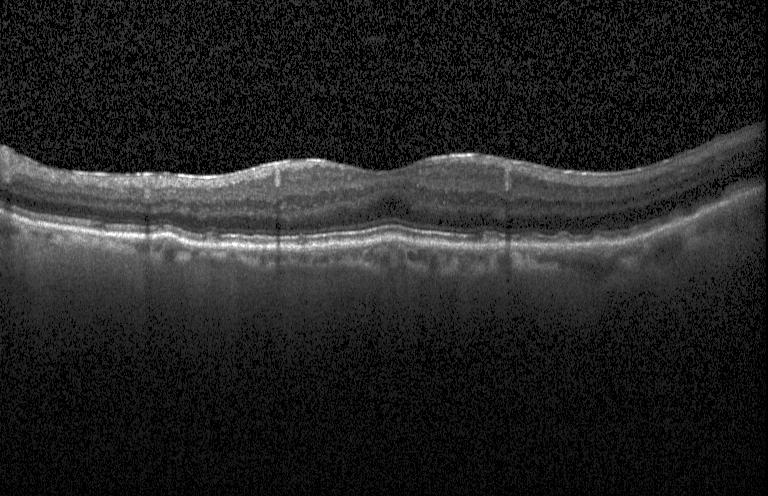

OCT line scan
Finding: multiple drusen.